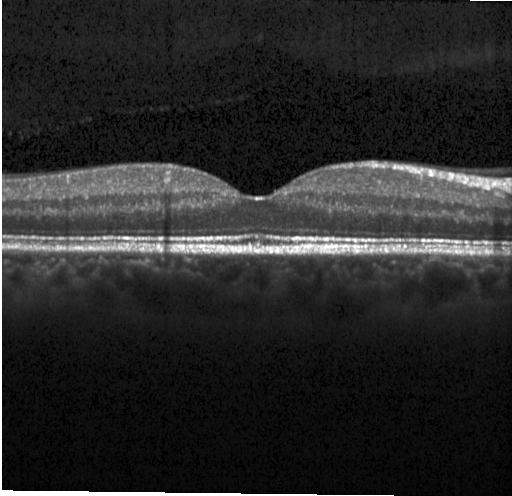 Fovea-centered. Heidelberg Spectralis. OCT B-scan. Impression: neither choroidal neovascularization, diabetic macular edema, nor drusen.